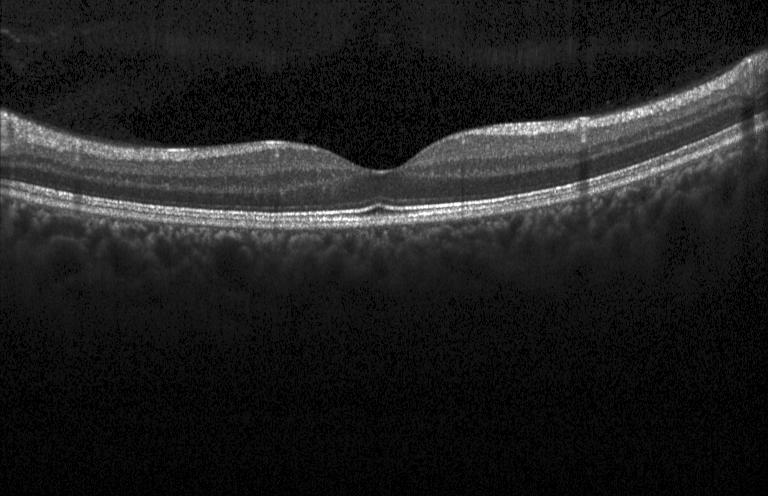
Spectral-domain OCT B-scan: no evidence of choroidal neovascularization, diabetic macular edema, or drusen.